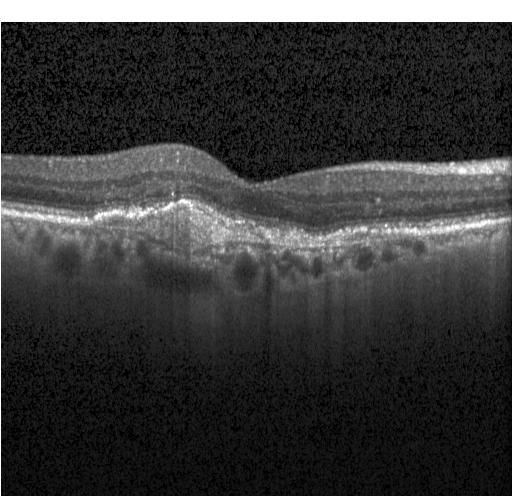

OCT B-scan showing a choroidal neovascular membrane.